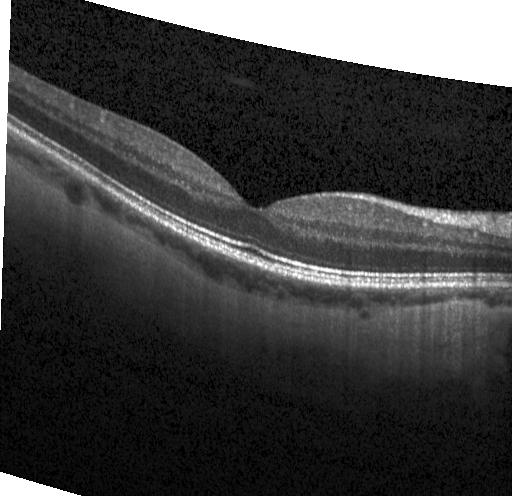 SD-OCT. Optical coherence tomography scan.
The scan shows no evidence of choroidal neovascularization, diabetic macular edema, or drusen.